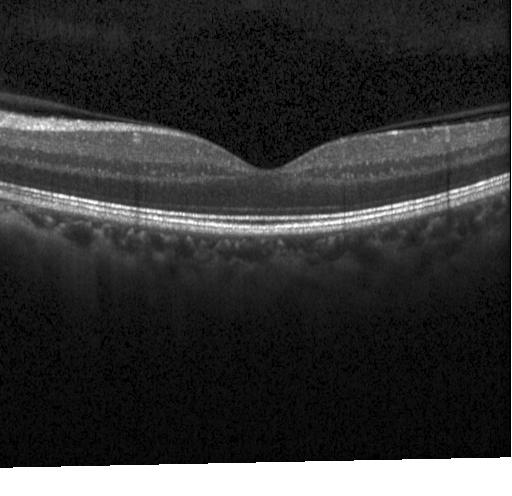 Spectral-domain OCT. Retinal OCT cross-section. Acquired on a Heidelberg Spectralis.
Diagnosis: no evidence of choroidal neovascularization, diabetic macular edema, or drusen.